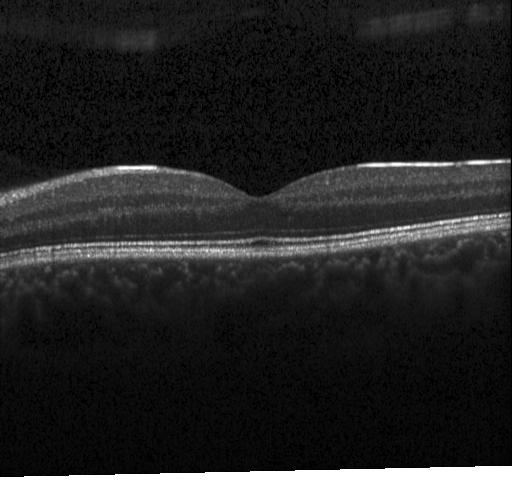

Impression: no choroidal neovascularization, diabetic macular edema, or drusen.